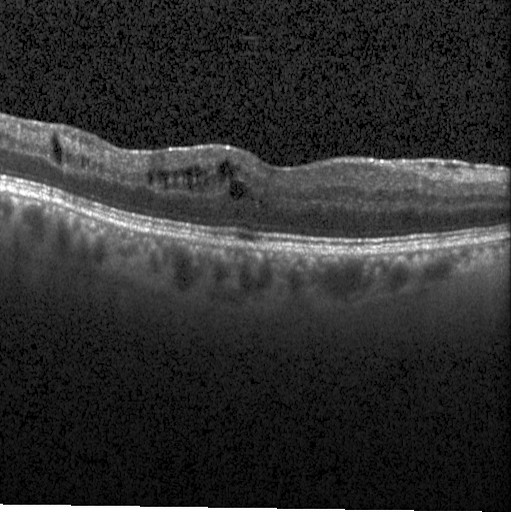
Finding: diabetic macular edema.